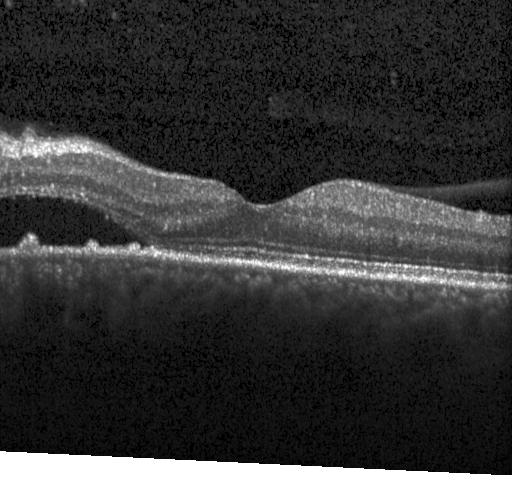 Retinal OCT cross-section.
Impression: choroidal neovascularization (CNV).